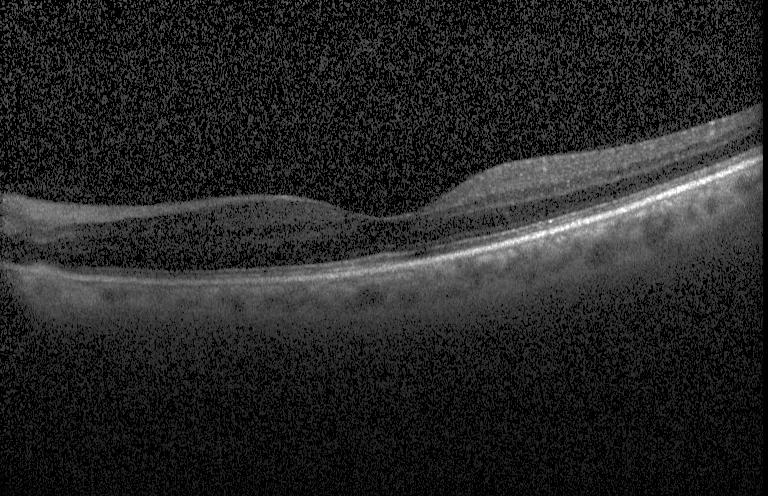

No evidence of choroidal neovascularization, diabetic macular edema, or drusen.